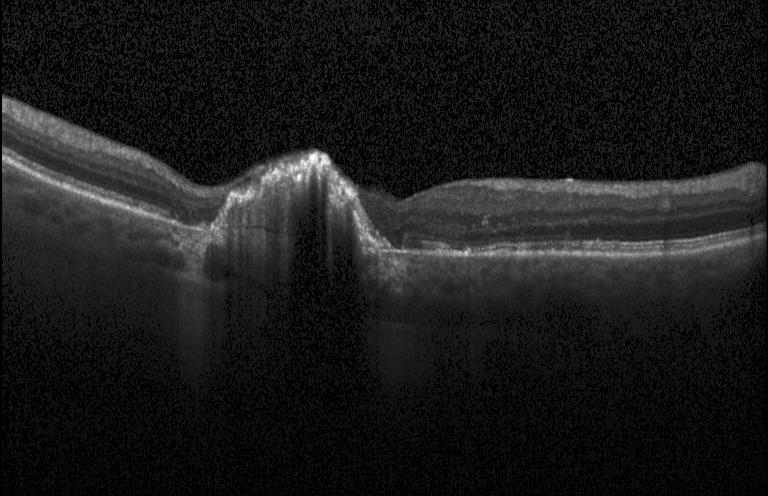

Fovea-centered; SD-OCT; OCT line scan — Finding: choroidal neovascularization.